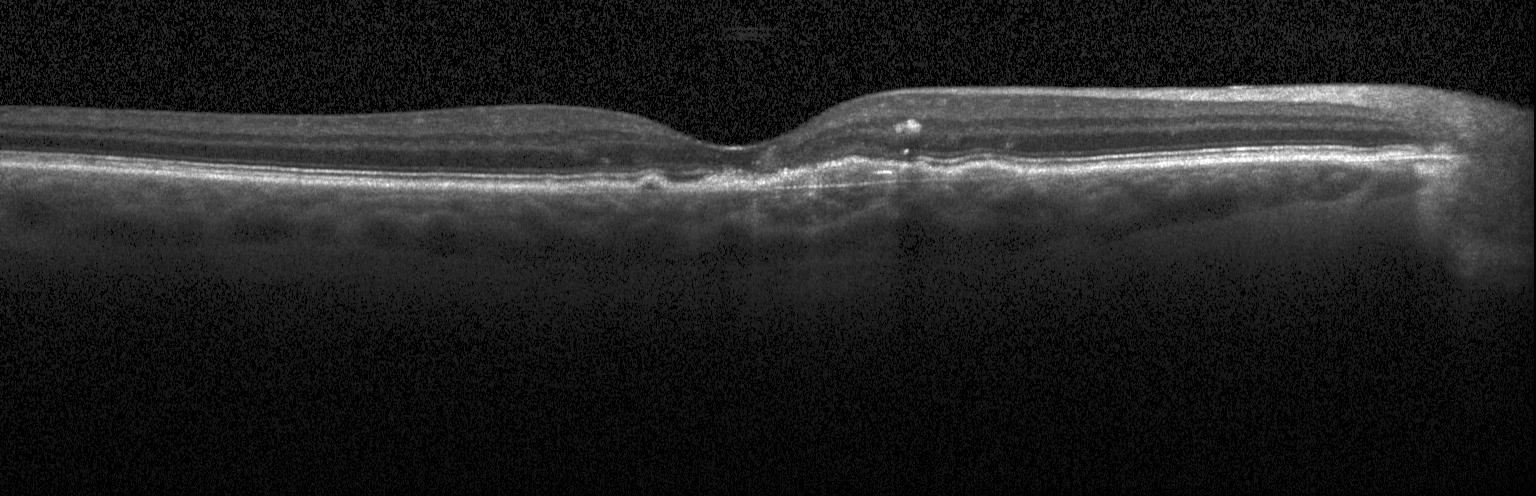
Macular OCT: a choroidal neovascular membrane.